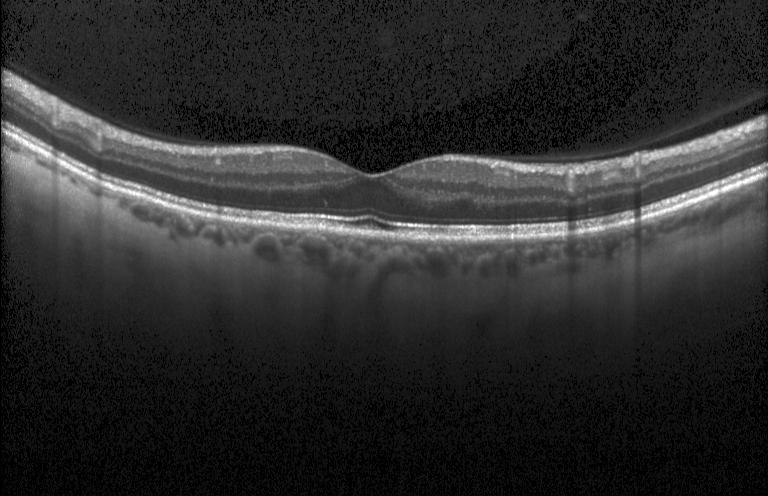

Spectral-domain optical coherence tomography. Optical coherence tomography B-scan — Dx: no evidence of CNV, DME, or drusen.